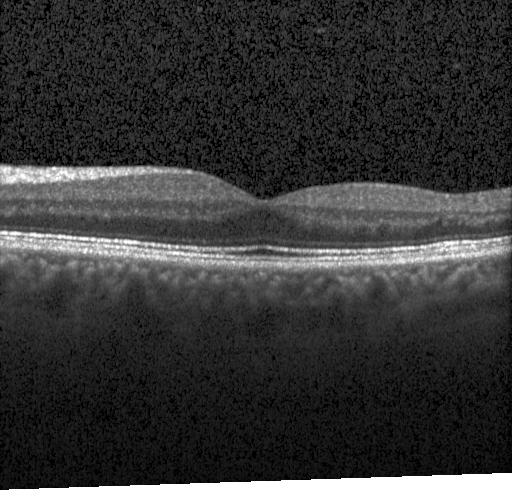
This B-scan demonstrates no choroidal neovascularization, diabetic macular edema, or drusen.